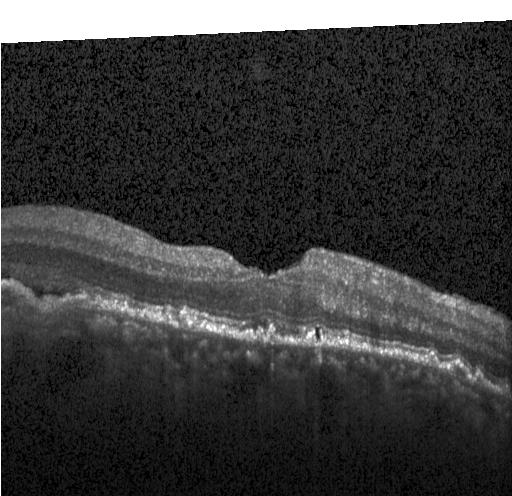

OCT line scan, acquired on a Heidelberg Spectralis, through the macula
Impression: a choroidal neovascular membrane.